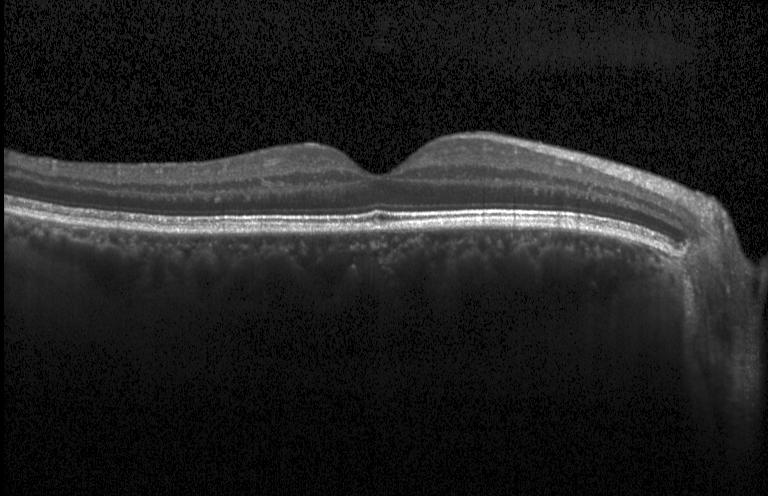
Instrument: Heidelberg Spectralis · OCT line scan · SD-OCT · horizontal scan through the fovea. Diagnosis: no choroidal neovascularization, diabetic macular edema, or drusen.